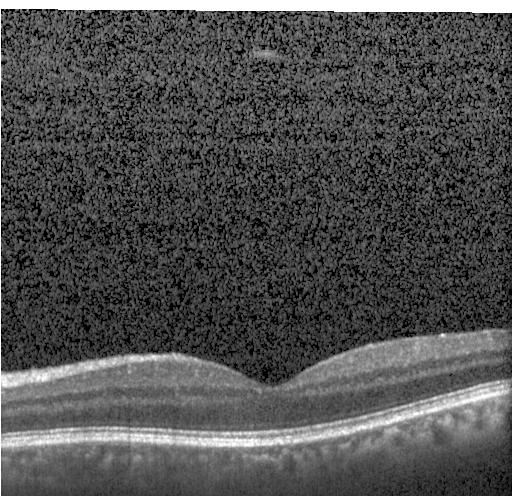 Diagnosis: neither choroidal neovascularization, diabetic macular edema, nor drusen.